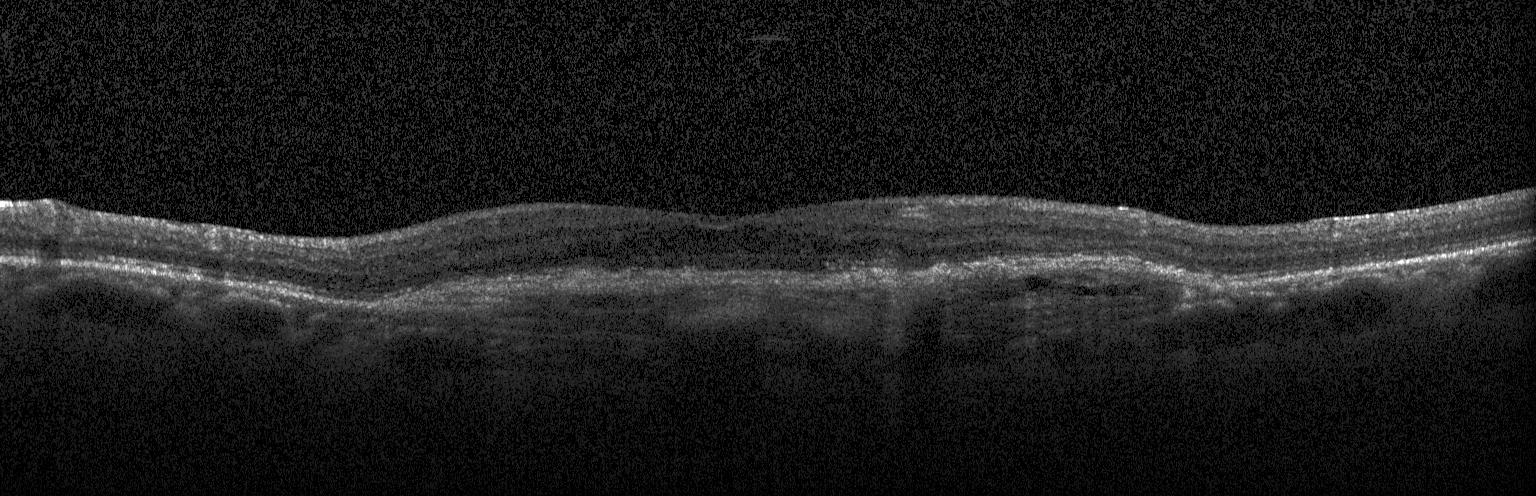 Impression: CNV.